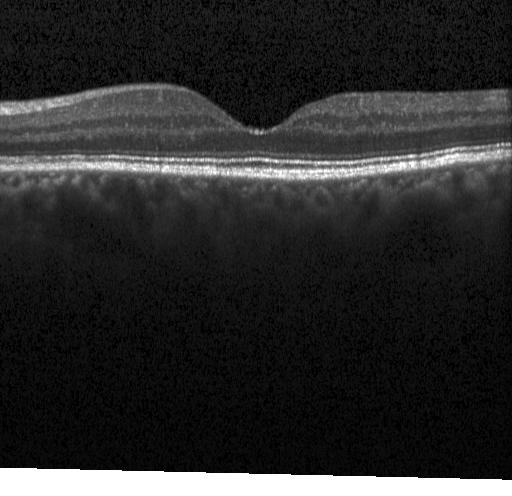

Spectral-domain OCT, instrument: Heidelberg Spectralis, optical coherence tomography B-scan, macular scan.
Finding: no evidence of CNV, DME, or drusen.